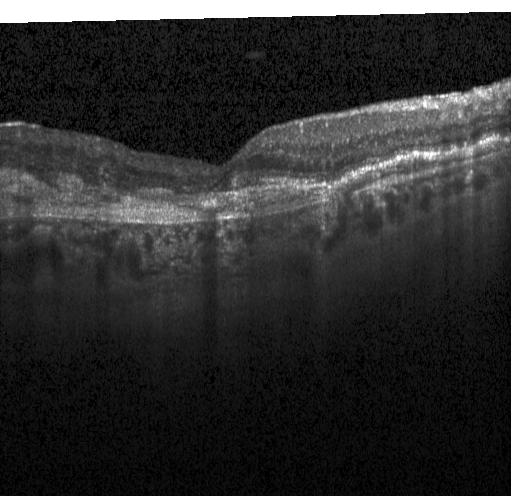

OCT finding: choroidal neovascularization (CNV).